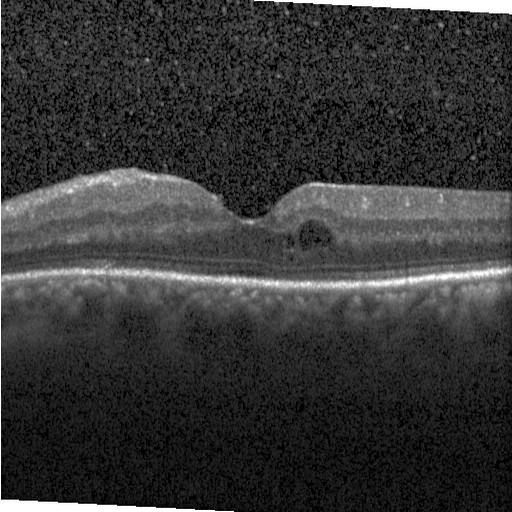
Optical coherence tomography scan. Finding: diabetic macular edema (DME).